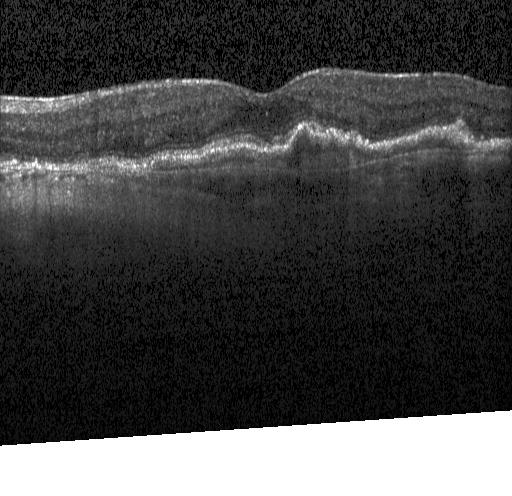

Diagnosis: choroidal neovascularization (CNV).